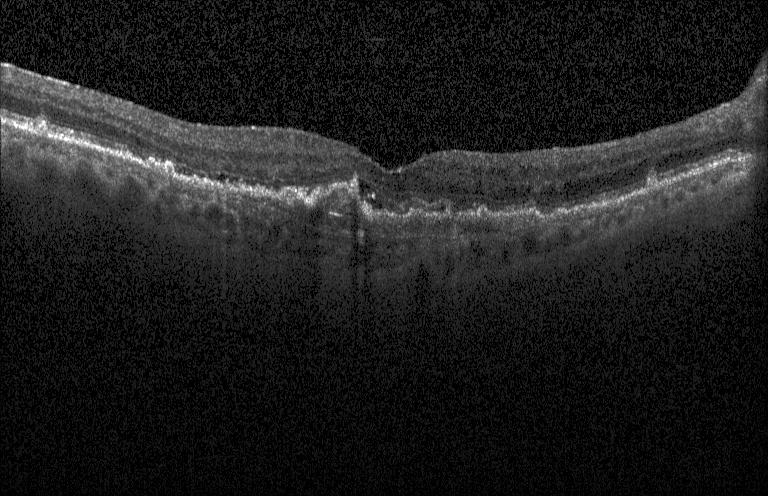 OCT line scan.
Diagnosis: a choroidal neovascular membrane.